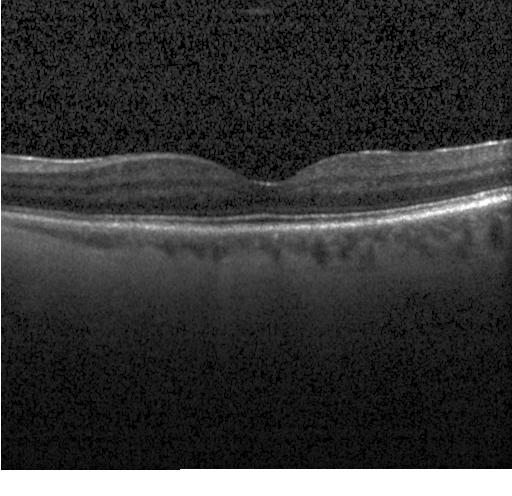

Retinal OCT cross-section showing no choroidal neovascularization, no diabetic macular edema, and no drusen.